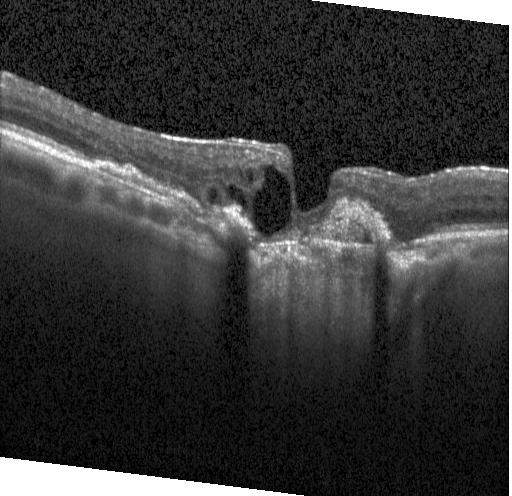

OCT B-scan showing a choroidal neovascular membrane.